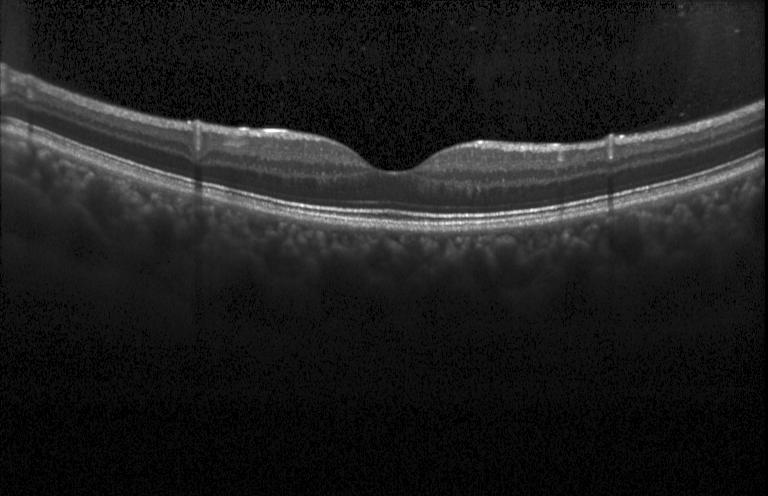
Finding: no choroidal neovascularization, diabetic macular edema, or drusen.